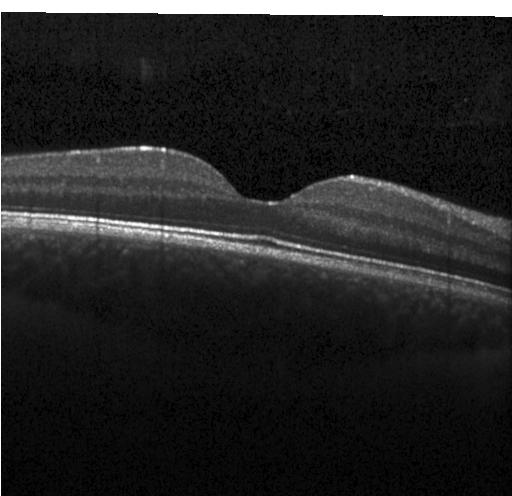 Retinal OCT cross-section — Impression: no choroidal neovascularization, diabetic macular edema, or drusen.